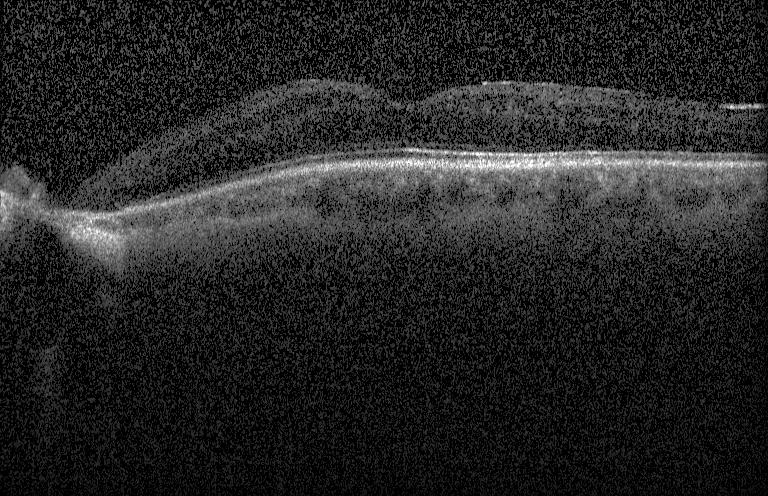
Optical coherence tomography B-scan; spectral-domain optical coherence tomography — Finding: no choroidal neovascularization, no diabetic macular edema, and no drusen.